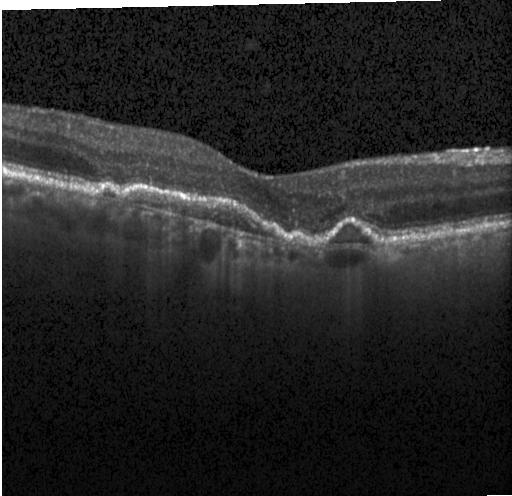
Macular OCT: a choroidal neovascular membrane.